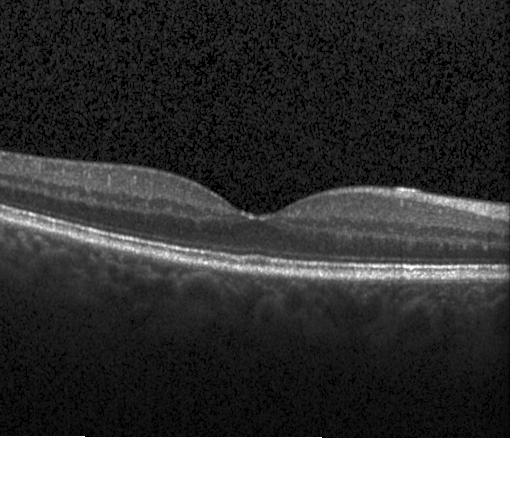
SD-OCT · retinal OCT B-scan · centered on the fovea · instrument: Heidelberg Spectralis
This B-scan demonstrates no CNV, no DME, and no drusen.